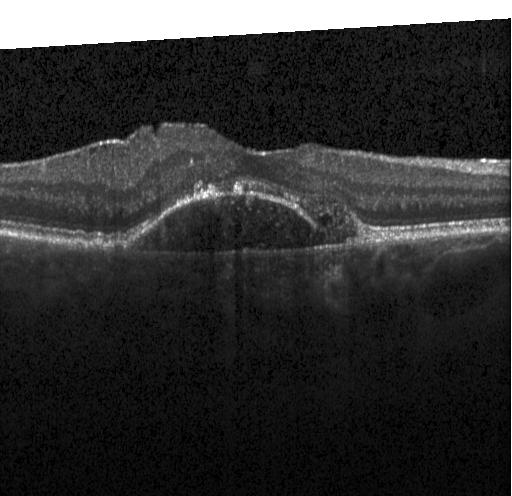

OCT line scan.
Diagnosis: a choroidal neovascular membrane.